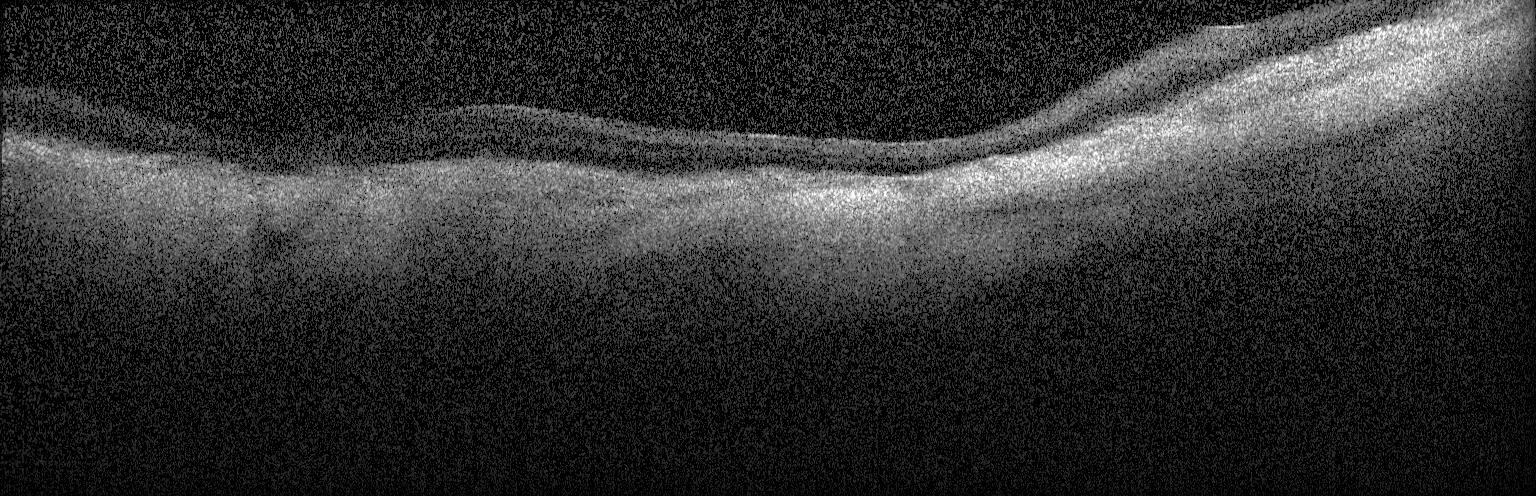

Diagnosis: CNV.